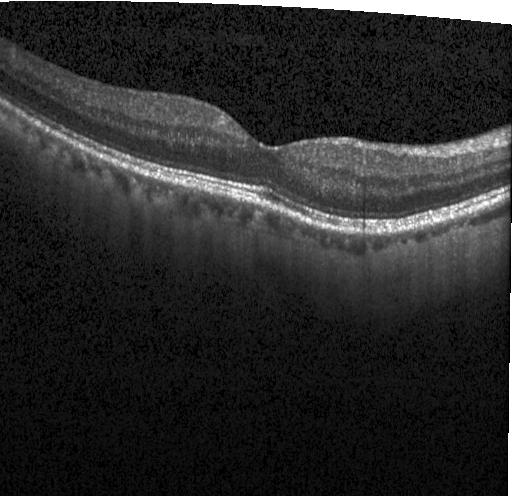
OCT B-scan, fovea-centered, spectral-domain OCT, Heidelberg Spectralis.
No evidence of choroidal neovascularization, diabetic macular edema, or drusen.